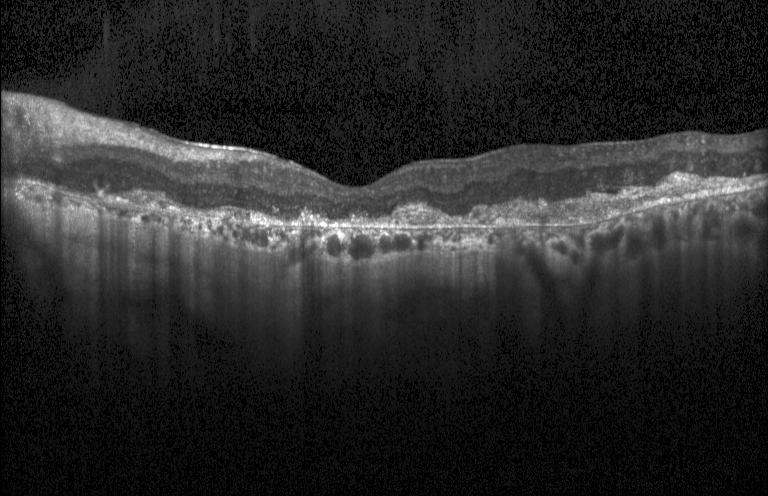
OCT B-scan; macular scan — Finding: choroidal neovascularization.